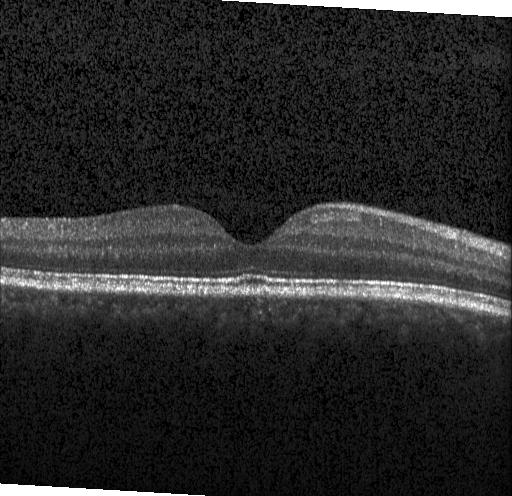

Instrument: Heidelberg Spectralis · optical coherence tomography scan. Macular OCT: no evidence of CNV, DME, or drusen.